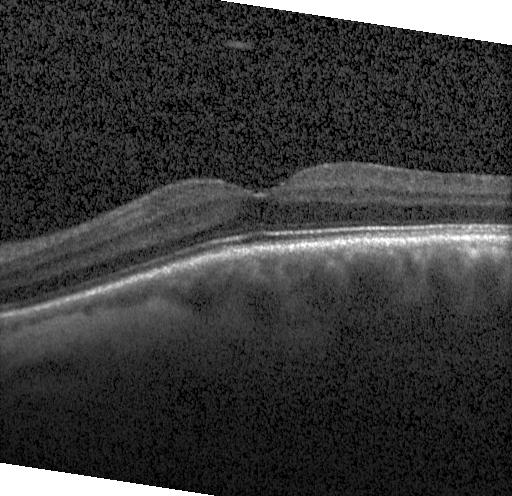

The scan shows neither choroidal neovascularization, diabetic macular edema, nor drusen.